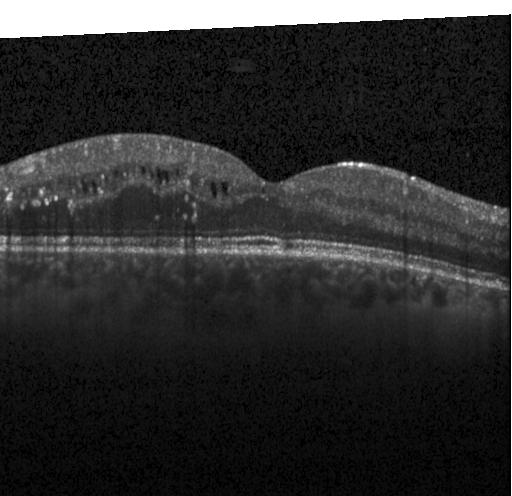

Retinal OCT cross-section.
The scan shows DME.